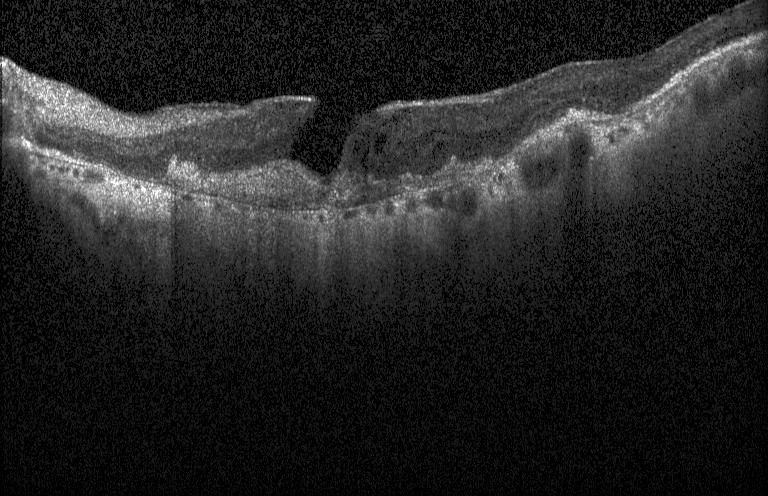 Impression: a choroidal neovascular membrane.